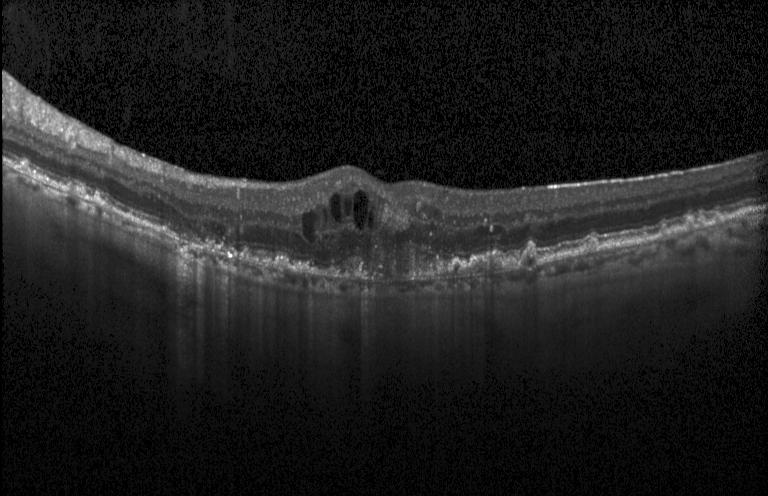 Diagnosis: choroidal neovascularization.